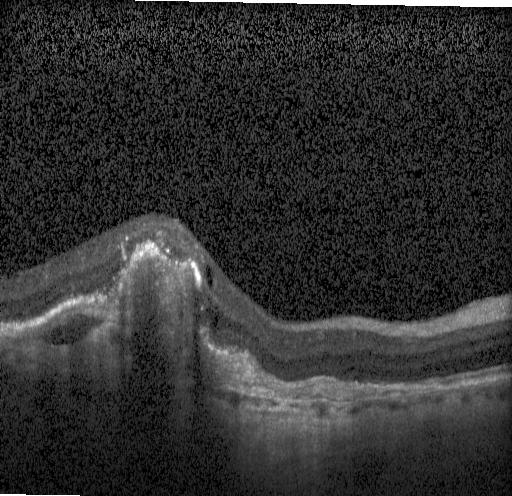
OCT B-scan showing a choroidal neovascular membrane.